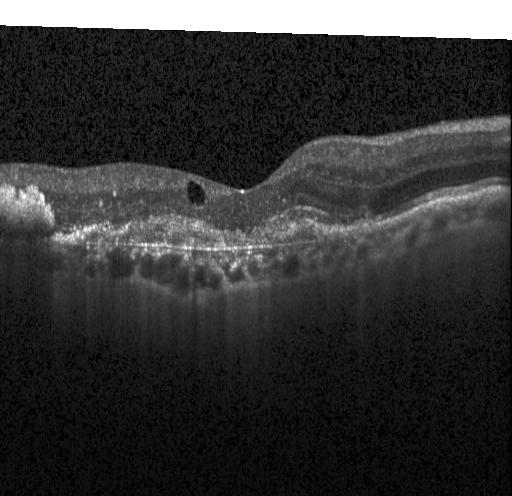
Heidelberg Spectralis OCT system, spectral-domain optical coherence tomography, centered on the fovea, optical coherence tomography B-scan — OCT finding: a choroidal neovascular membrane.